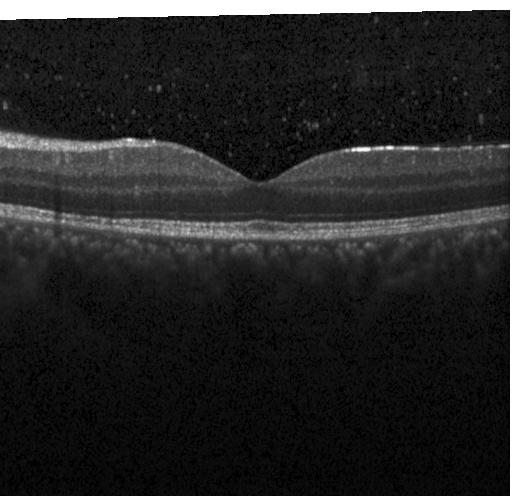 Finding: no evidence of CNV, DME, or drusen.